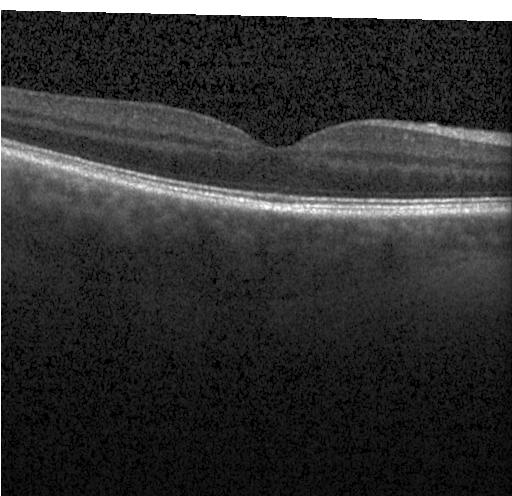
Macular OCT demonstrating no evidence of CNV, DME, or drusen.